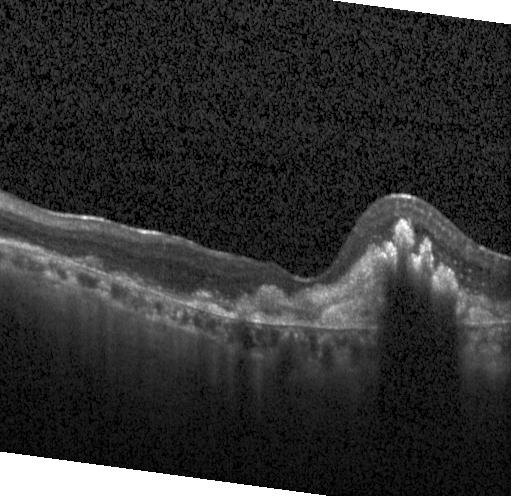

Retinal OCT B-scan, SD-OCT. Macular OCT: choroidal neovascularization.